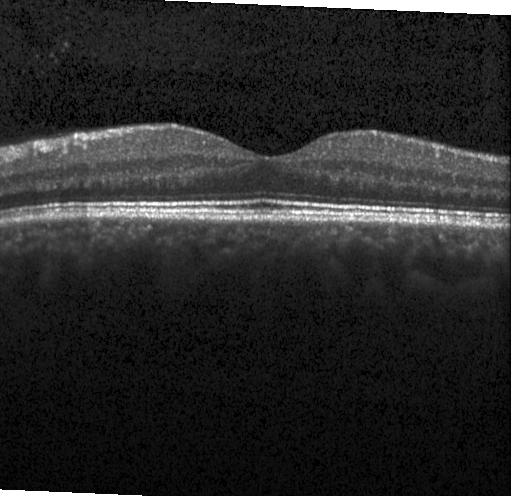 Retinal OCT cross-section — The scan shows neither choroidal neovascularization, diabetic macular edema, nor drusen.